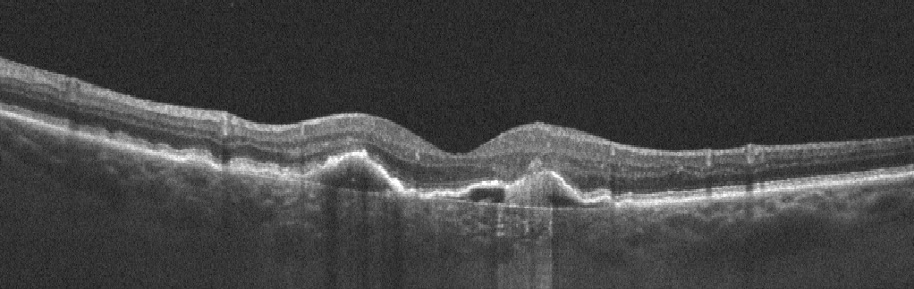

AMD.